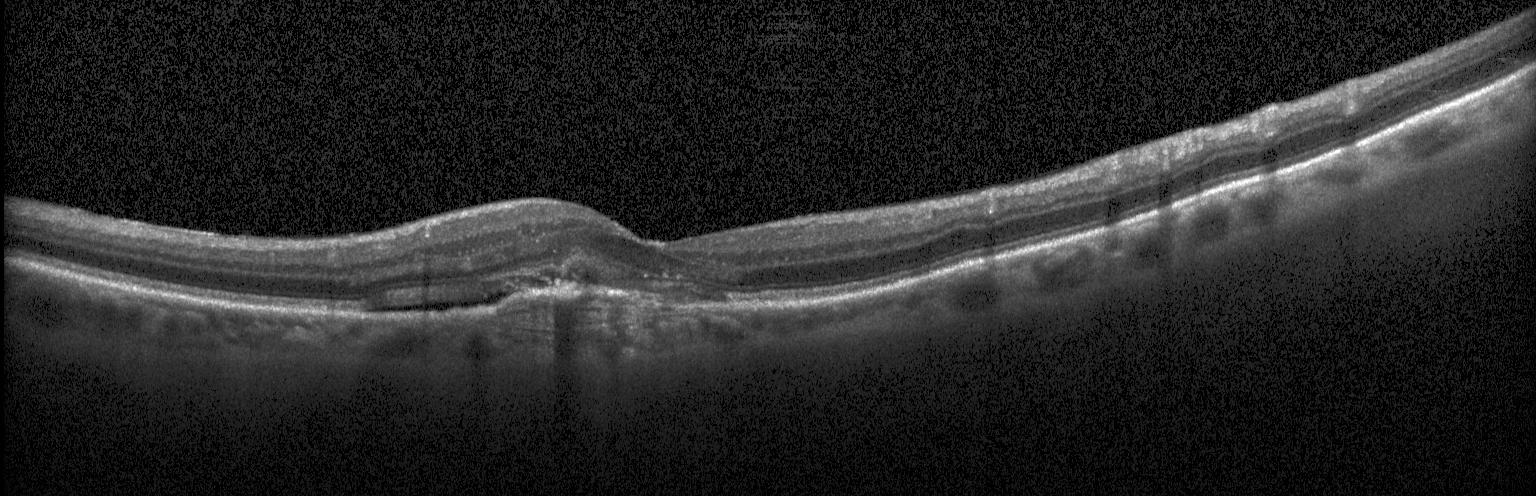
This B-scan demonstrates a choroidal neovascular membrane.